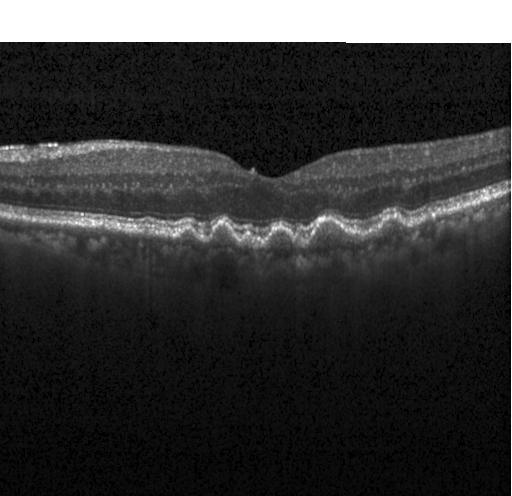

Retinal OCT cross-section showing multiple drusen.